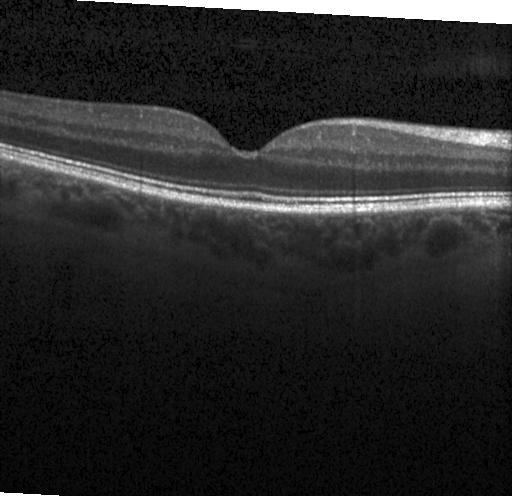 Finding: neither choroidal neovascularization, diabetic macular edema, nor drusen.